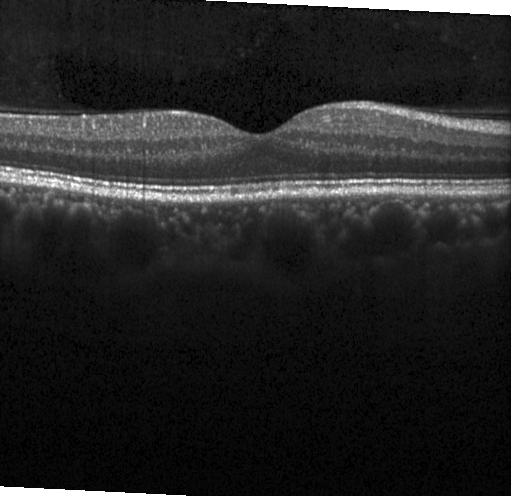 Centered on the fovea · retinal OCT cross-section · spectral-domain OCT · Heidelberg Spectralis OCT system
This B-scan demonstrates no evidence of CNV, DME, or drusen.